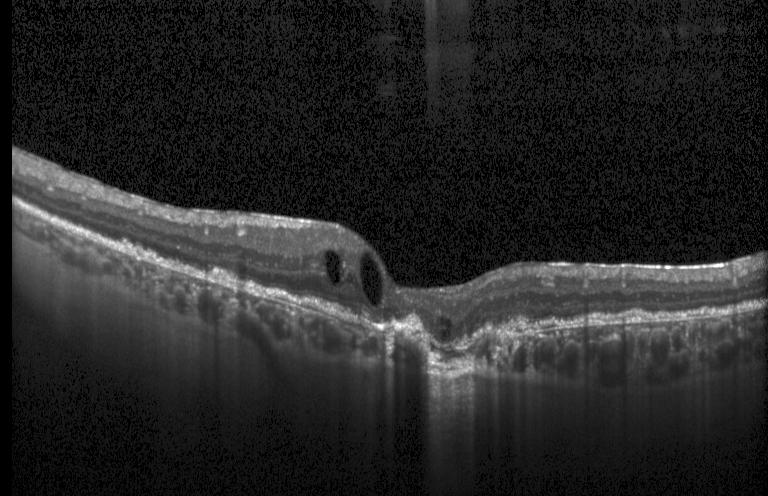

Optical coherence tomography scan. Impression: a choroidal neovascular membrane.